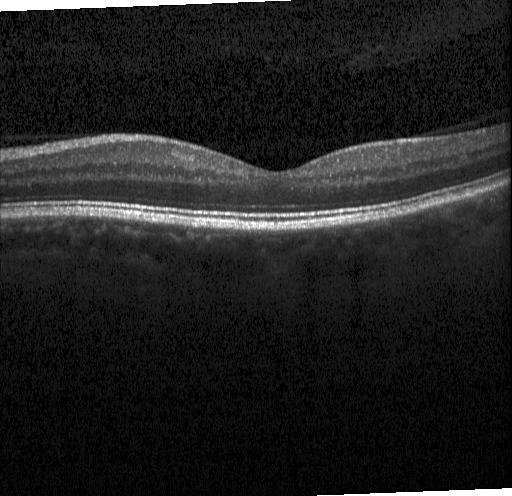

Optical coherence tomography B-scan — Macular OCT: no choroidal neovascularization, no diabetic macular edema, and no drusen.